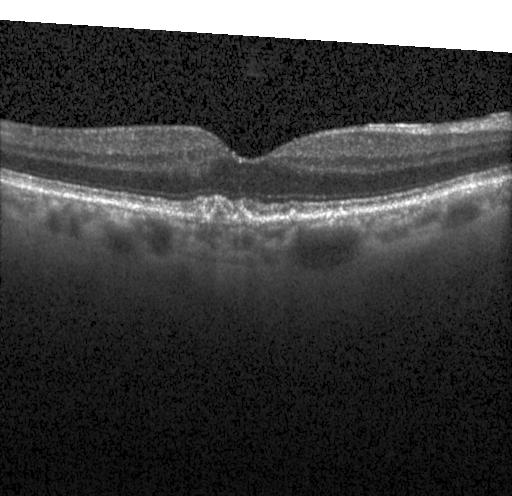

Fovea-centered, OCT B-scan, Heidelberg Spectralis.
Impression: sub-RPE drusenoid deposits.